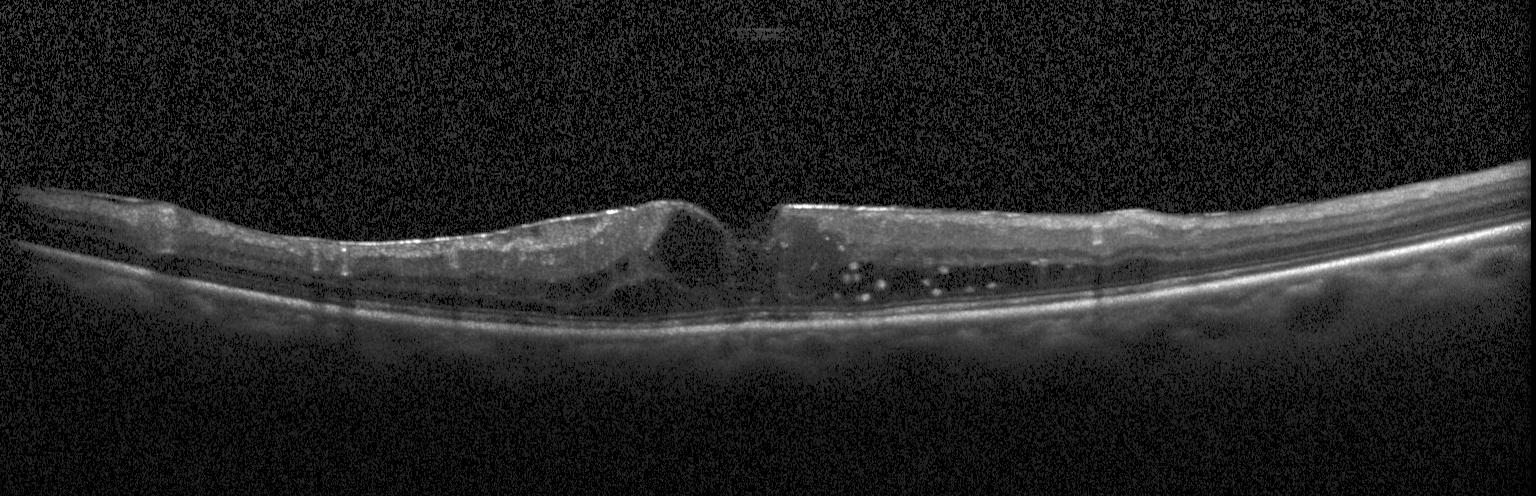
Through the macula · retinal OCT B-scan. Finding: diabetic macular edema (DME).